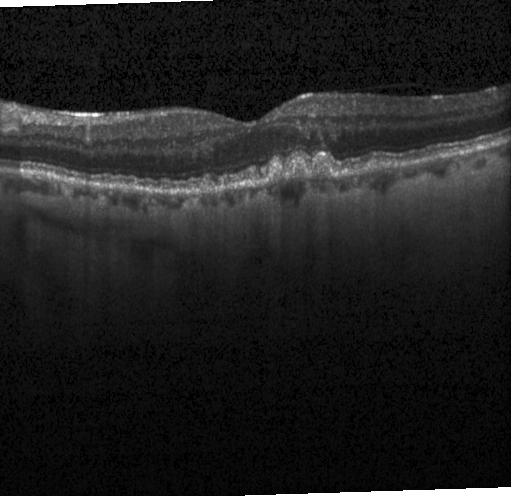
Dx: drusen.